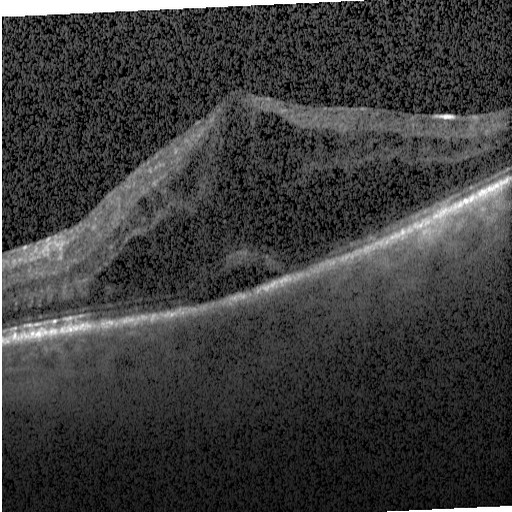

Through the macula; SD-OCT; OCT line scan.
Impression: DME.